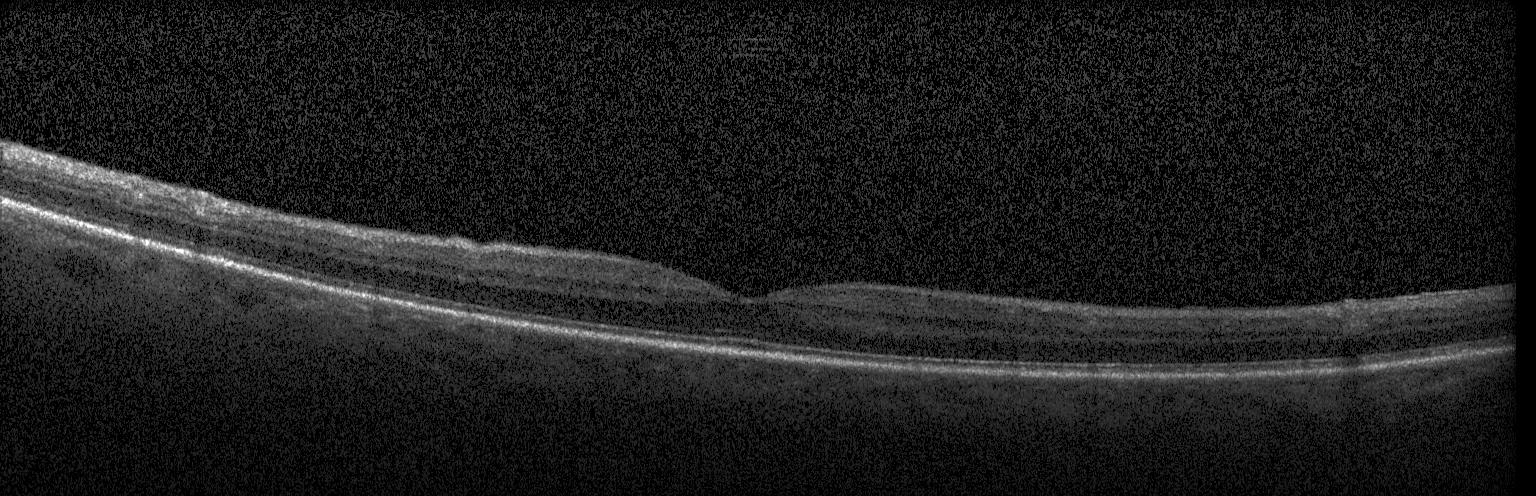

This B-scan demonstrates neither choroidal neovascularization, diabetic macular edema, nor drusen.